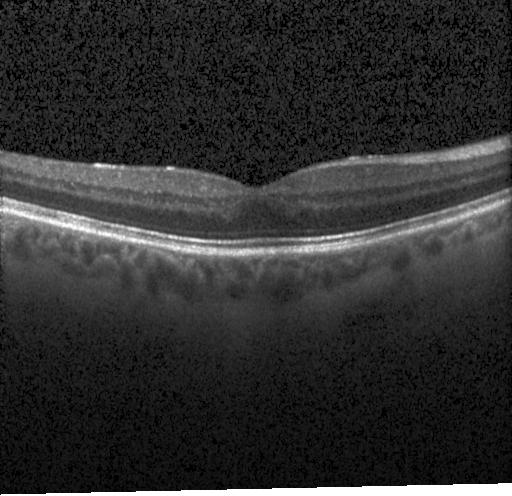
Dx: no choroidal neovascularization, no diabetic macular edema, and no drusen.